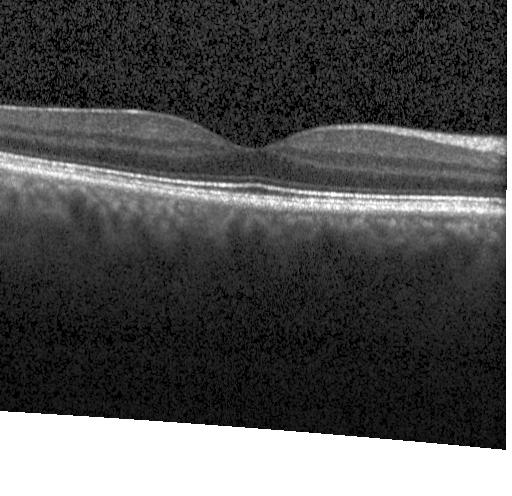
Horizontal scan through the fovea. Heidelberg Spectralis. Spectral-domain OCT. OCT line scan — Dx: neither CNV, DME, nor drusen.